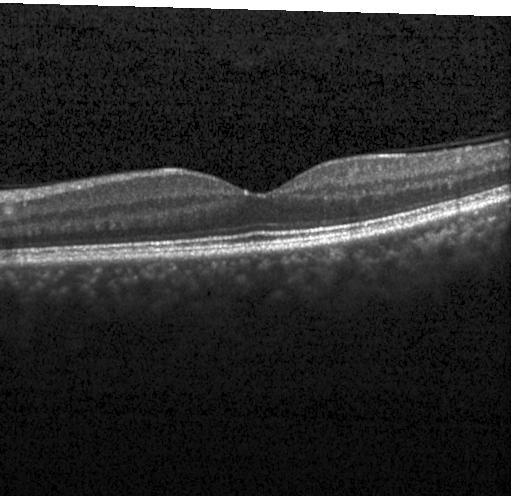 OCT line scan; spectral-domain OCT; fovea-centered. Dx: no evidence of choroidal neovascularization, diabetic macular edema, or drusen.